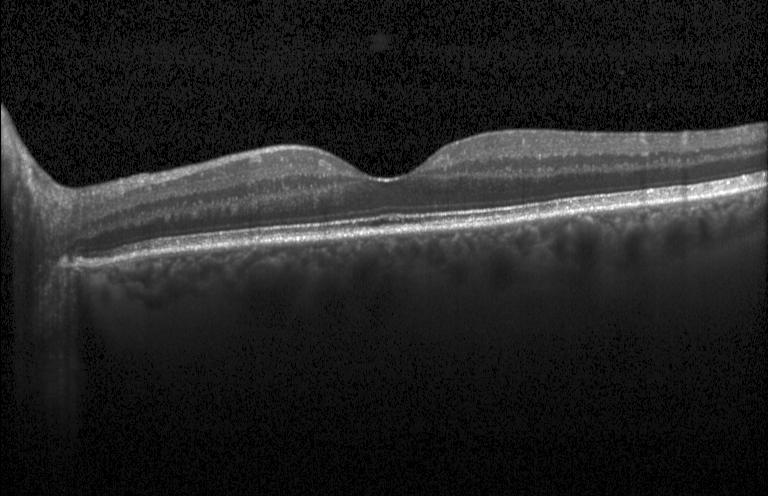
This B-scan demonstrates no evidence of CNV, DME, or drusen.